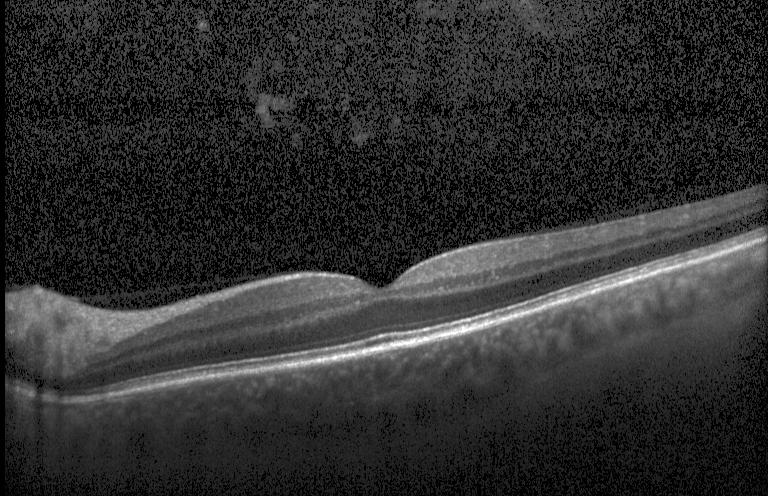
Acquired on a Heidelberg Spectralis. Through the macula. Optical coherence tomography B-scan. Spectral-domain OCT
Dx: neither choroidal neovascularization, diabetic macular edema, nor drusen.